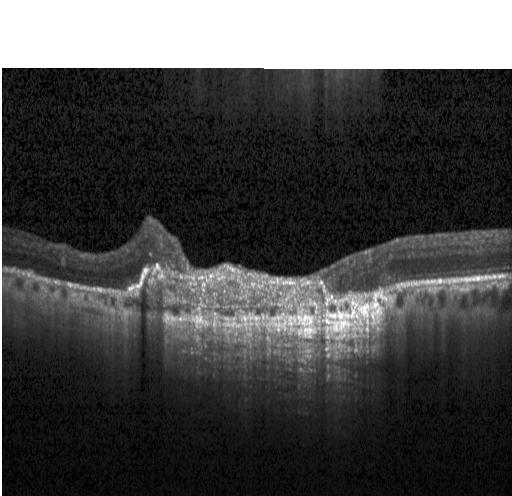

Macular scan; OCT B-scan; spectral-domain optical coherence tomography; instrument: Heidelberg Spectralis — Dx: a choroidal neovascular membrane.